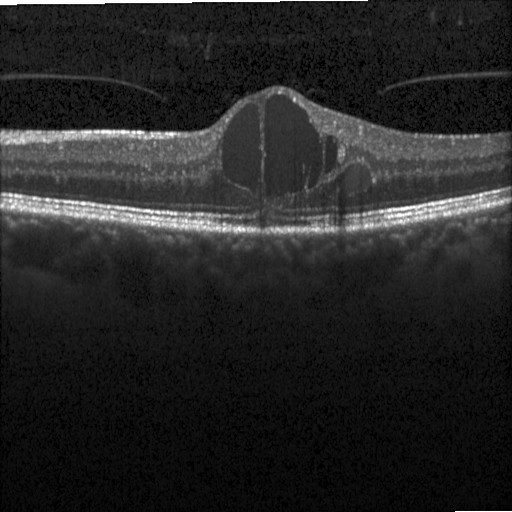
Impression: diabetic macular edema.